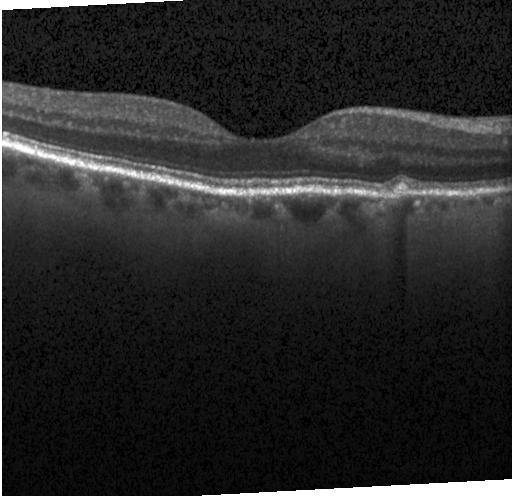
Instrument: Heidelberg Spectralis, centered on the fovea, OCT B-scan — This B-scan demonstrates multiple drusen.